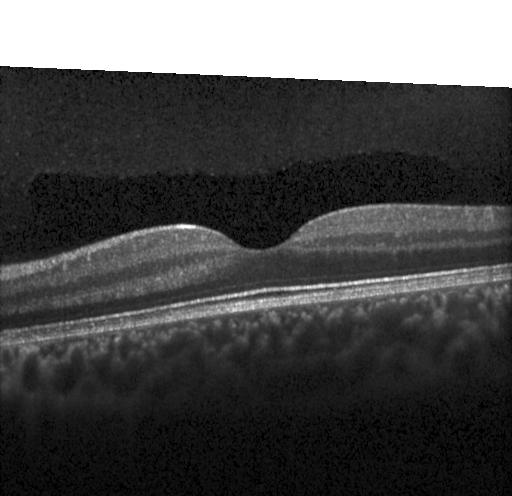
Dx: neither CNV, DME, nor drusen.